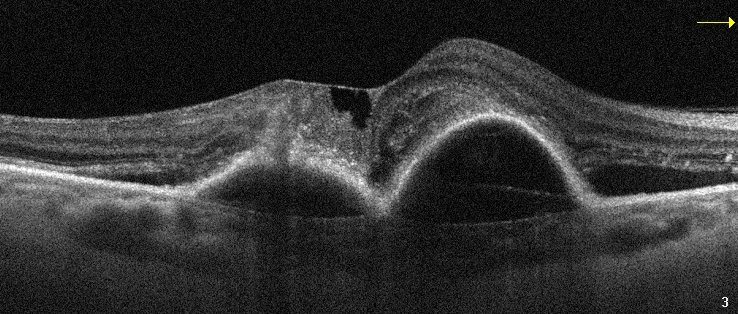

Retinal OCT cross-section
Impression: age-related macular degeneration (AMD).